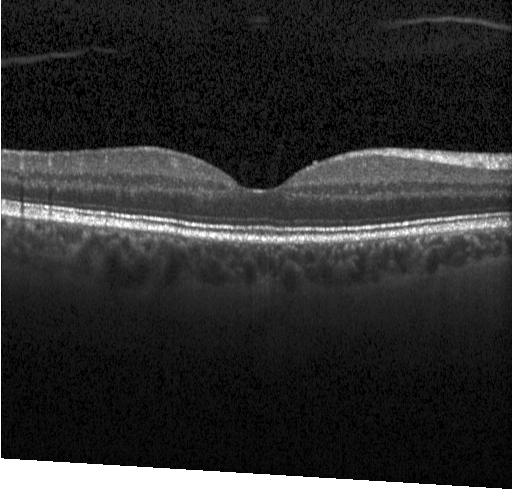 Retinal OCT B-scan · instrument: Heidelberg Spectralis
Impression: neither CNV, DME, nor drusen.